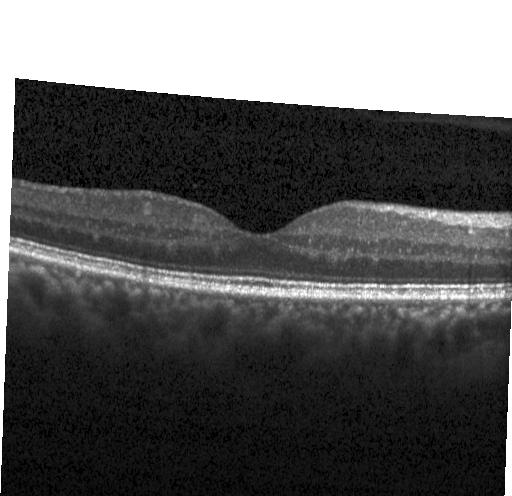

Horizontal scan through the fovea. Instrument: Heidelberg Spectralis. OCT B-scan
Impression: no choroidal neovascularization, no diabetic macular edema, and no drusen.